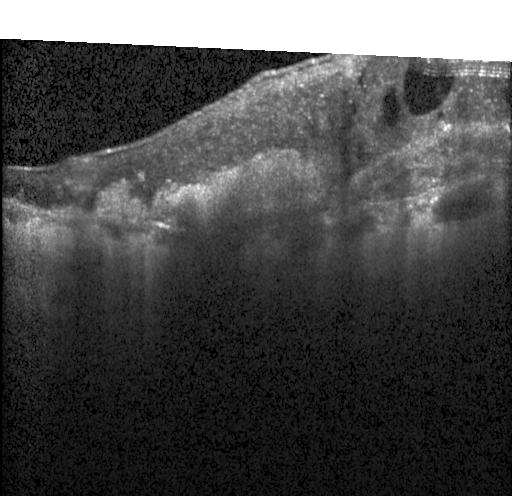 Macular scan; spectral-domain OCT; retinal OCT cross-section.
Finding: a choroidal neovascular membrane.